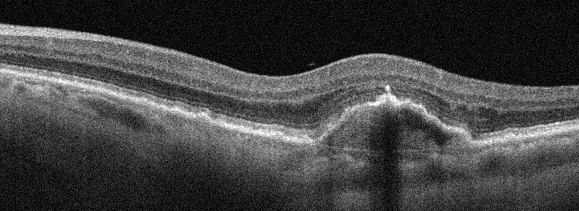

OCT B-scan. OS
Impression: AMD.